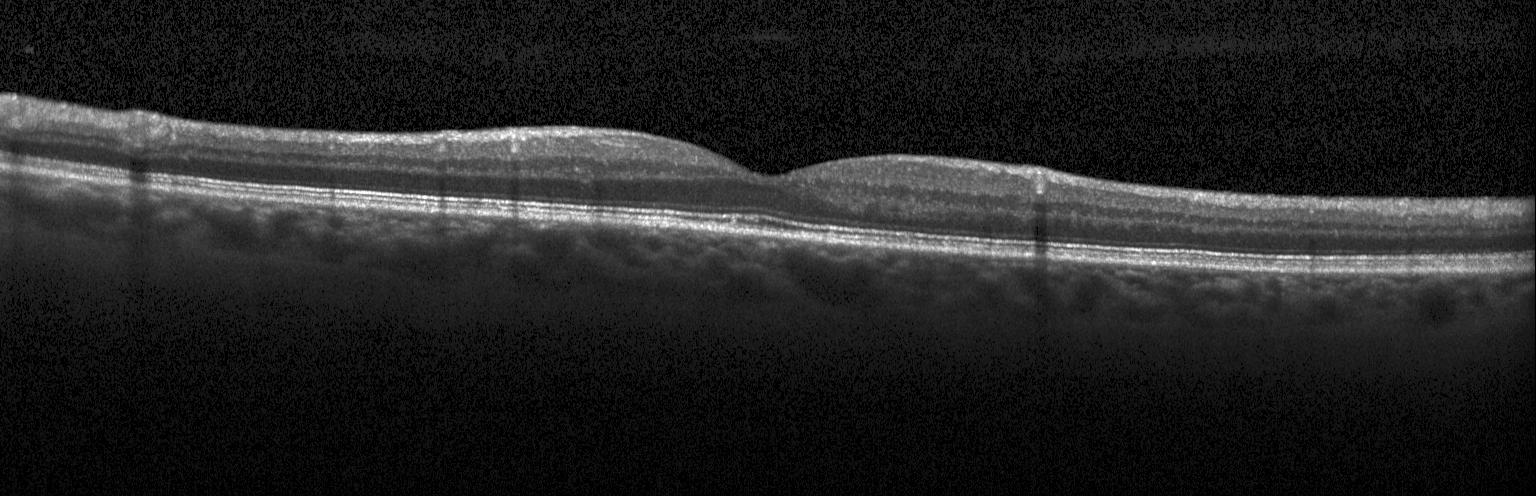

Retinal OCT cross-section; Heidelberg Spectralis; centered on the fovea; SD-OCT. Diagnosis: no choroidal neovascularization, no diabetic macular edema, and no drusen.